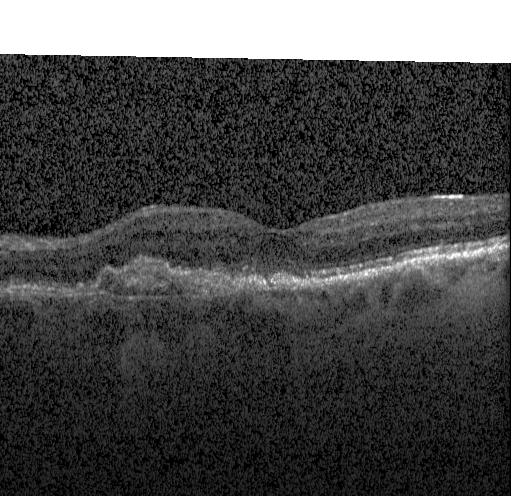
Impression: choroidal neovascularization (CNV).